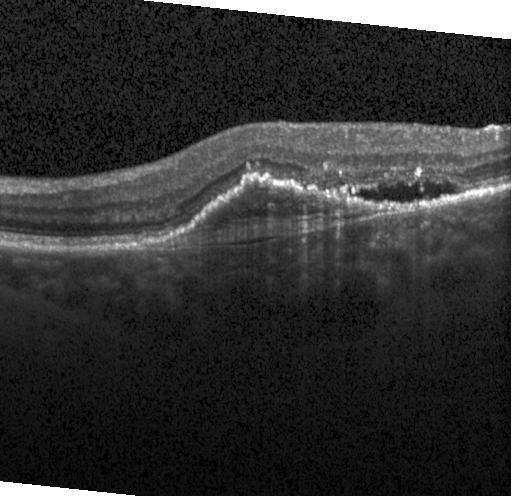

Heidelberg Spectralis OCT system; optical coherence tomography B-scan.
Impression: a choroidal neovascular membrane.